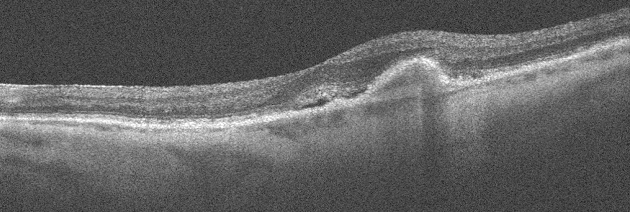 Acquired on an Optovue Avanti RTVue XR · retinal OCT B-scan · through the macula · OS. Impression: age-related macular degeneration (AMD).